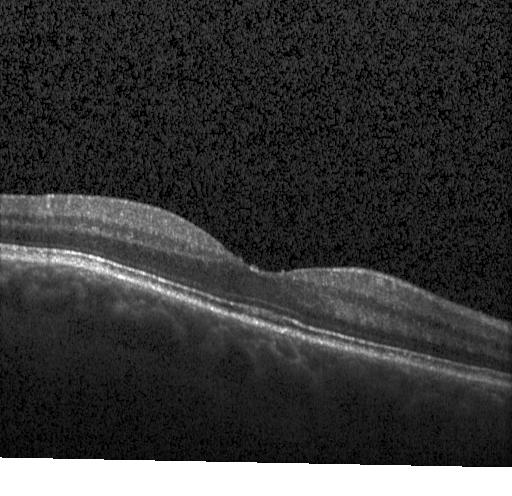

Impression: no choroidal neovascularization, diabetic macular edema, or drusen.